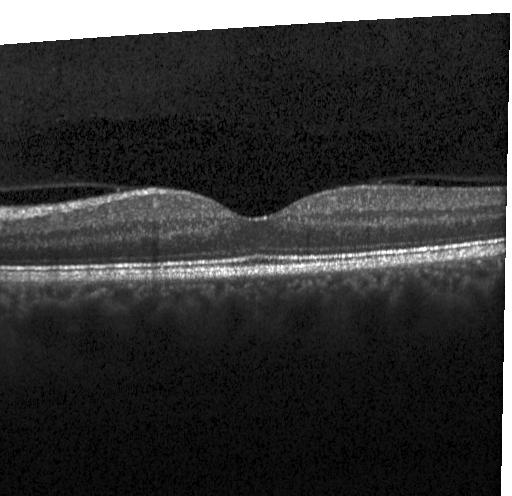
Macular OCT demonstrating no choroidal neovascularization, no diabetic macular edema, and no drusen.